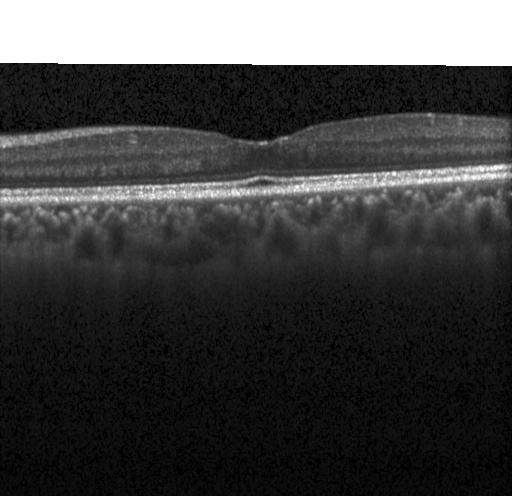 Spectral-domain OCT, retinal OCT cross-section, acquired on a Heidelberg Spectralis
Diagnosis: no choroidal neovascularization, diabetic macular edema, or drusen.